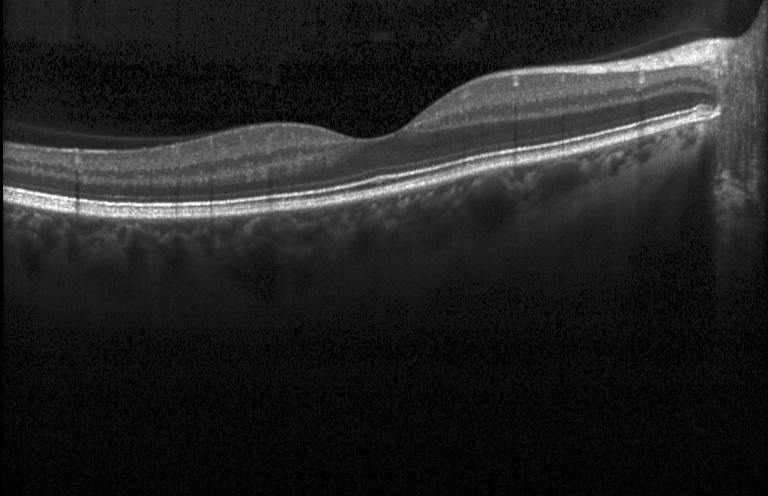

Impression: no CNV, DME, or drusen.